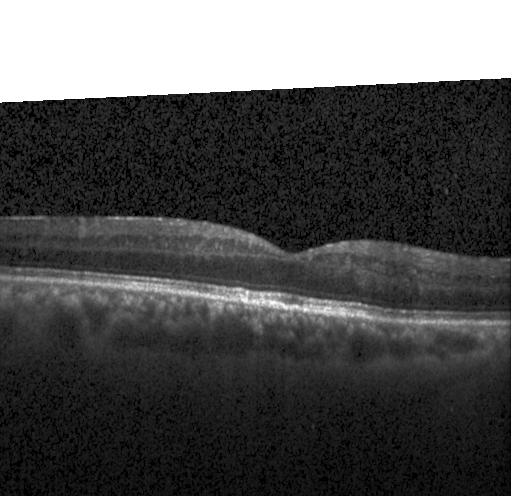
Dx: no choroidal neovascularization, diabetic macular edema, or drusen.